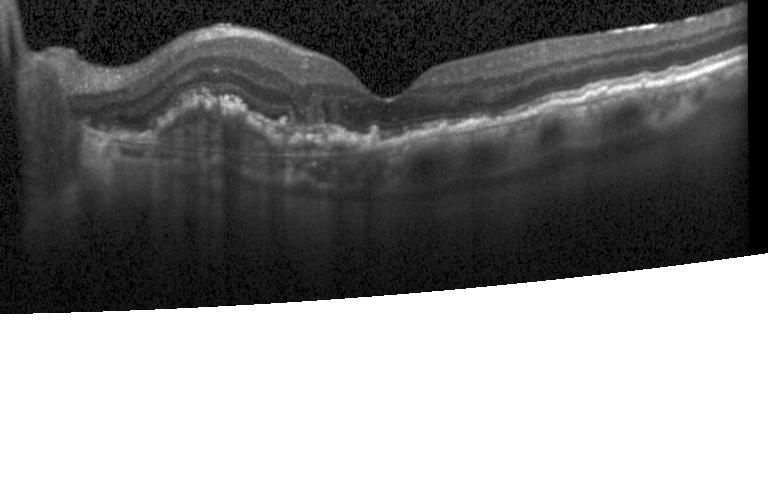 Retinal OCT cross-section
OCT finding: a choroidal neovascular membrane.